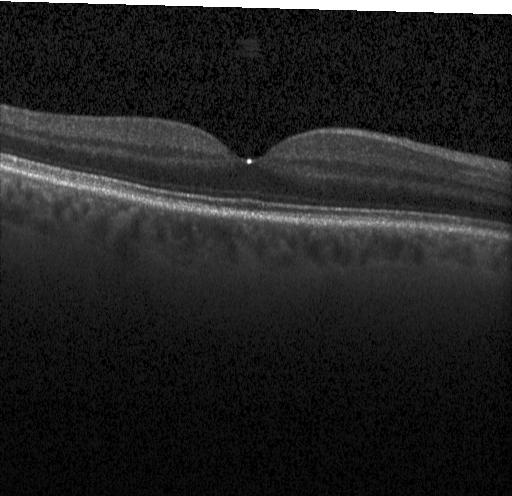
Dx: no choroidal neovascularization, no diabetic macular edema, and no drusen.